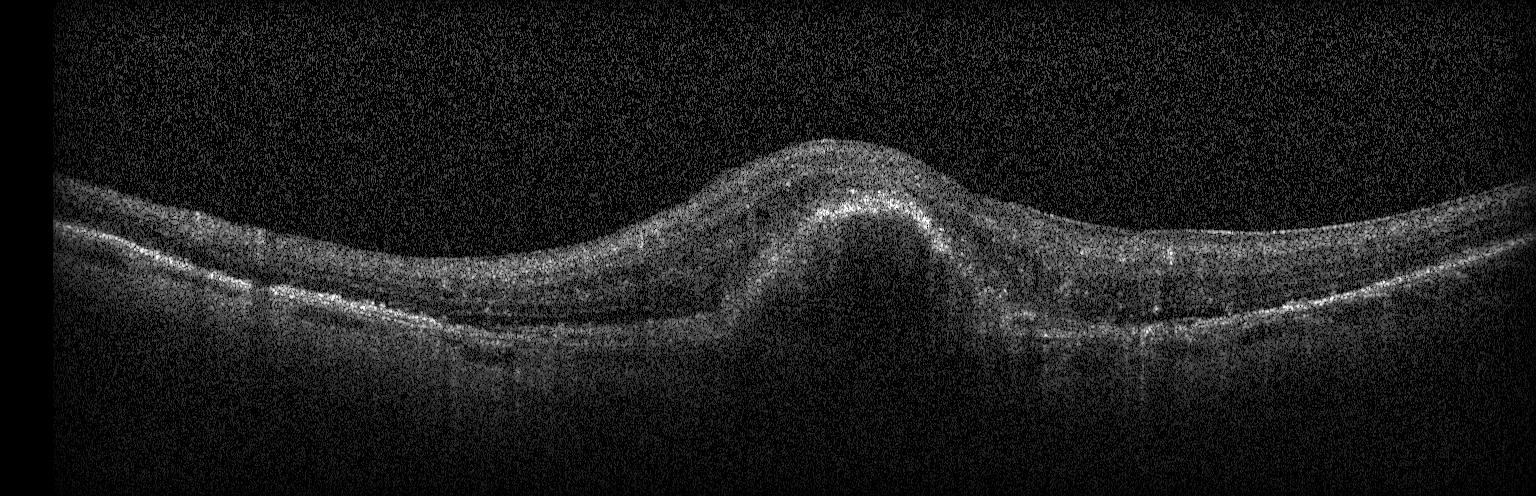
Diagnosis: CNV.